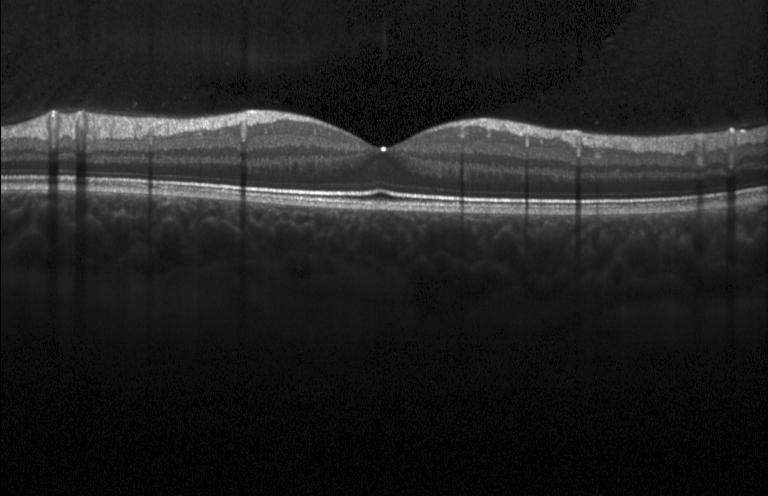
Optical coherence tomography scan. Horizontal scan through the fovea.
Impression: no choroidal neovascularization, no diabetic macular edema, and no drusen.